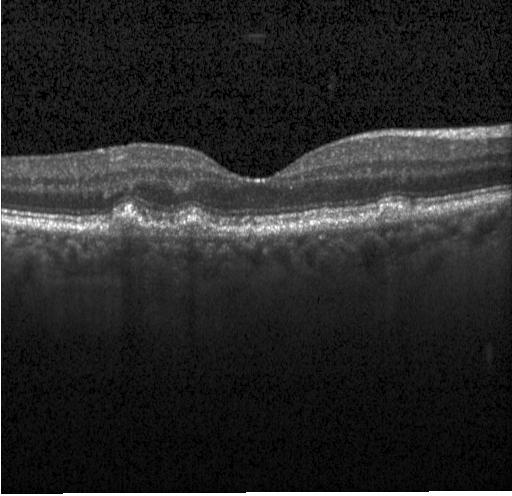 Spectral-domain OCT. Horizontal scan through the fovea. Retinal OCT B-scan. Heidelberg Spectralis. Diagnosis: sub-RPE drusenoid deposits.